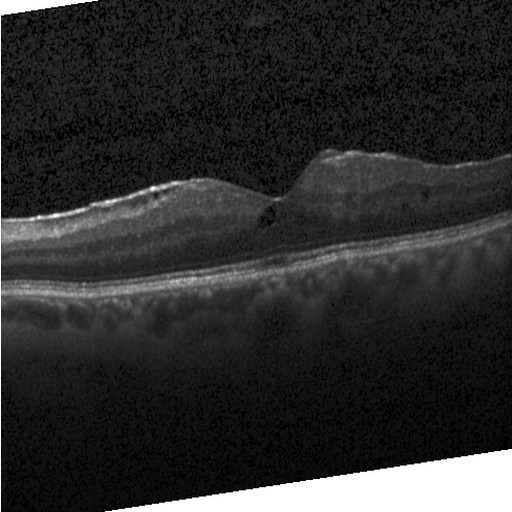

Optical coherence tomography B-scan · acquired on a Heidelberg Spectralis — Impression: diabetic macular edema (DME).